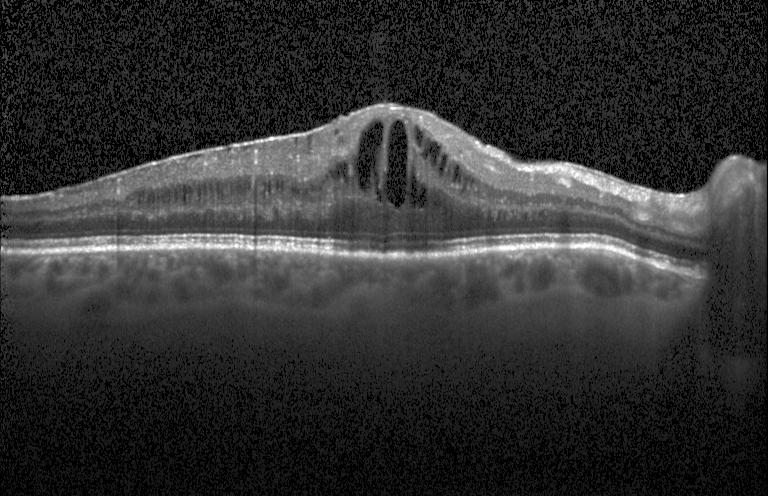 Macular OCT demonstrating DME.